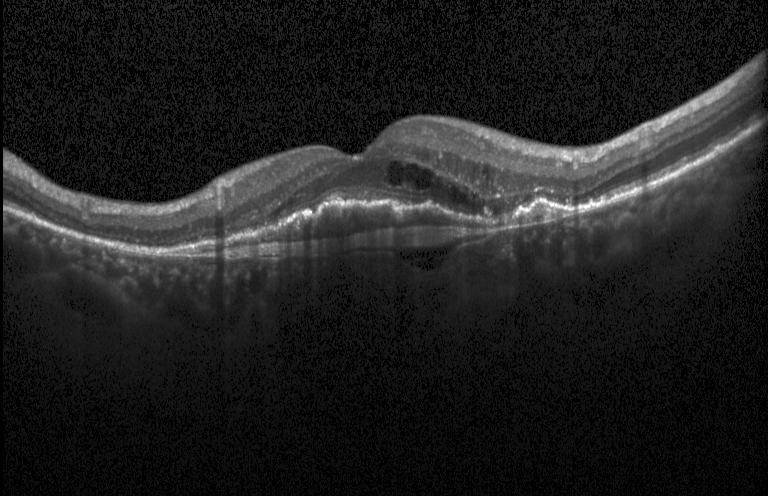

Dx: choroidal neovascularization (CNV).